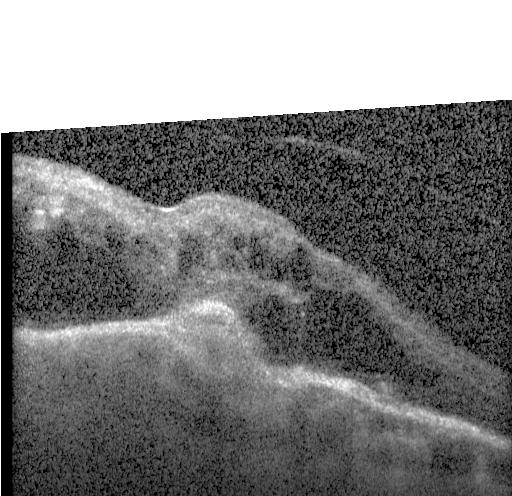

Impression: a choroidal neovascular membrane.